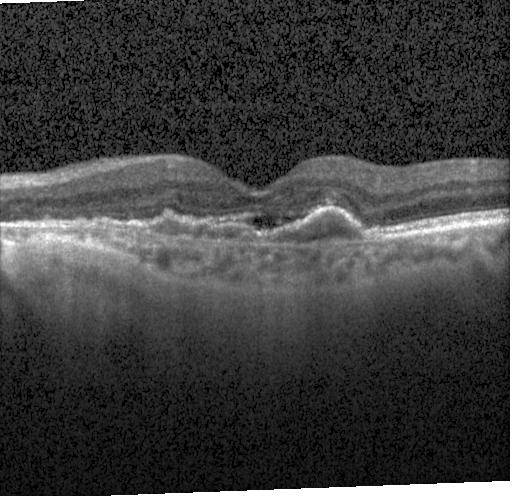
Acquired on a Heidelberg Spectralis; OCT line scan; spectral-domain OCT; centered on the fovea. Impression: CNV.